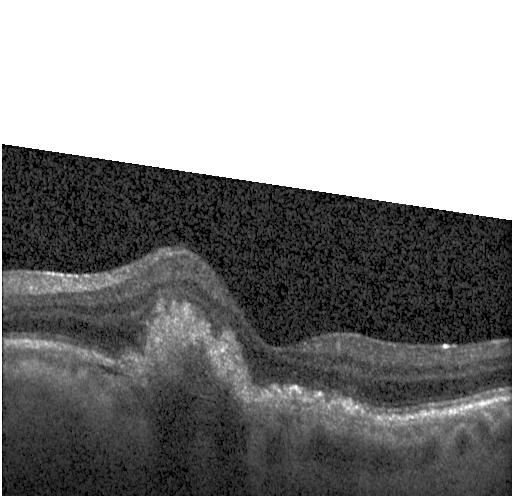

Optical coherence tomography scan. Macular OCT: choroidal neovascularization (CNV).